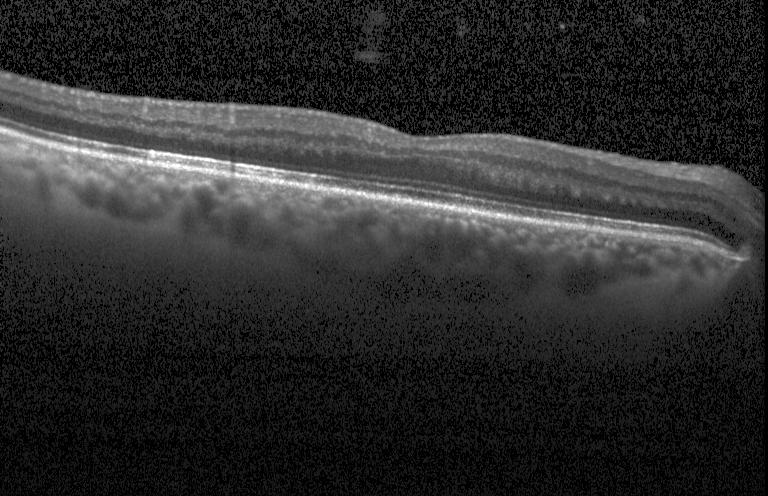

OCT line scan — OCT finding: no choroidal neovascularization, diabetic macular edema, or drusen.